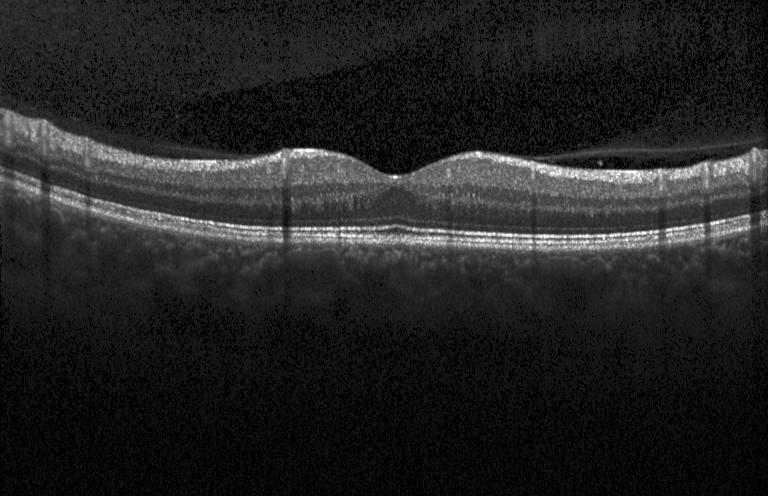 Retinal OCT cross-section. Spectral-domain OCT. Heidelberg Spectralis OCT system
Assessment: neither choroidal neovascularization, diabetic macular edema, nor drusen.